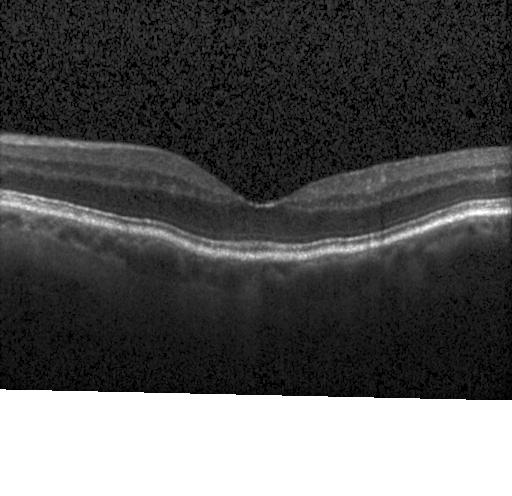 Finding: no evidence of choroidal neovascularization, diabetic macular edema, or drusen.